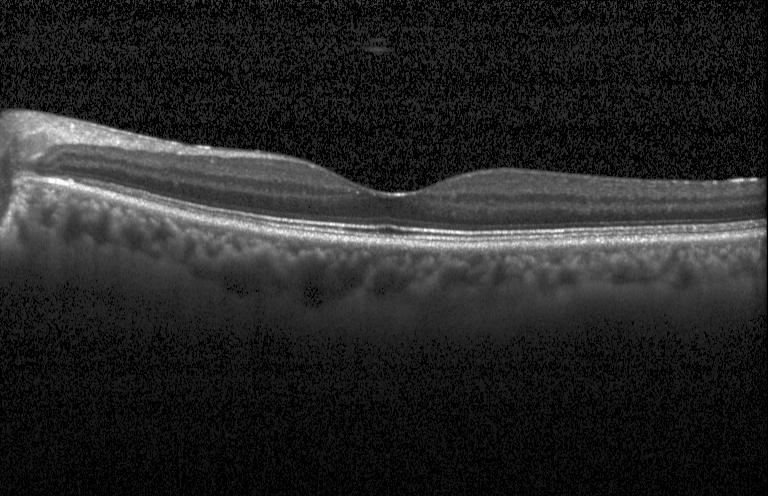
OCT finding: no choroidal neovascularization, diabetic macular edema, or drusen.